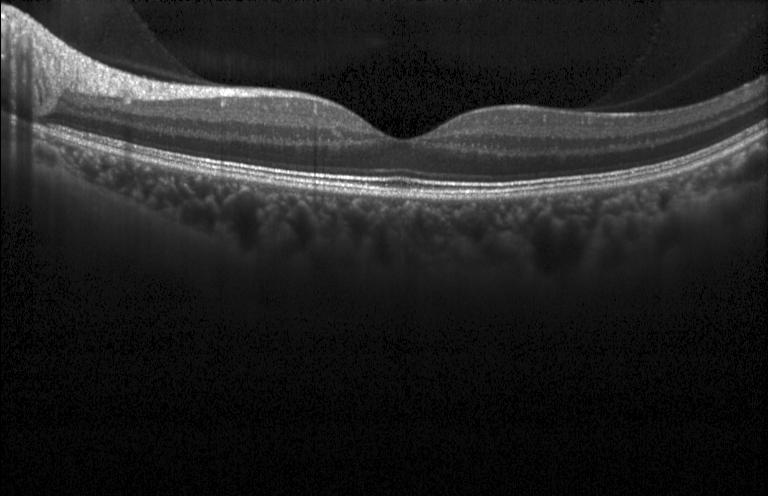

Optical coherence tomography scan
Neither choroidal neovascularization, diabetic macular edema, nor drusen.